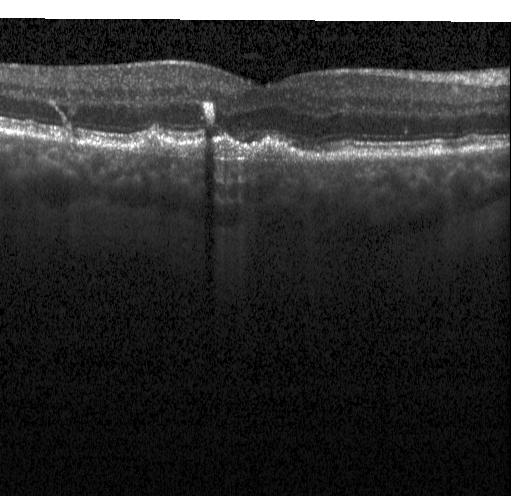

Optical coherence tomography B-scan · acquired on a Heidelberg Spectralis · macular scan. This B-scan demonstrates choroidal neovascularization (CNV).